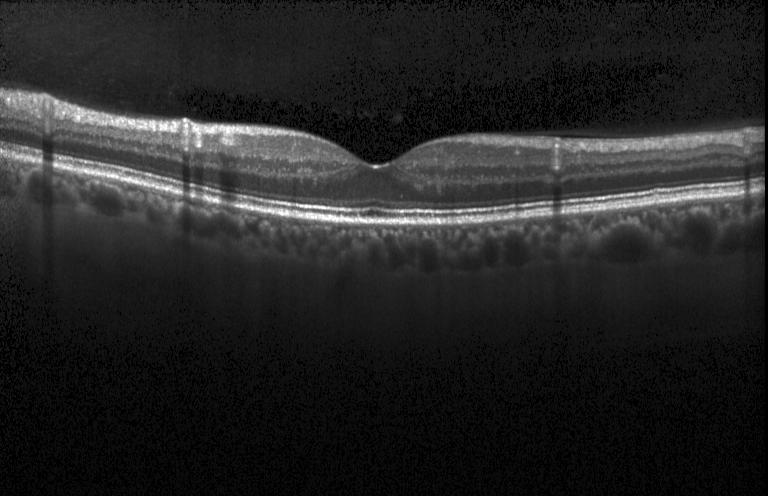
Impression: no evidence of choroidal neovascularization, diabetic macular edema, or drusen.